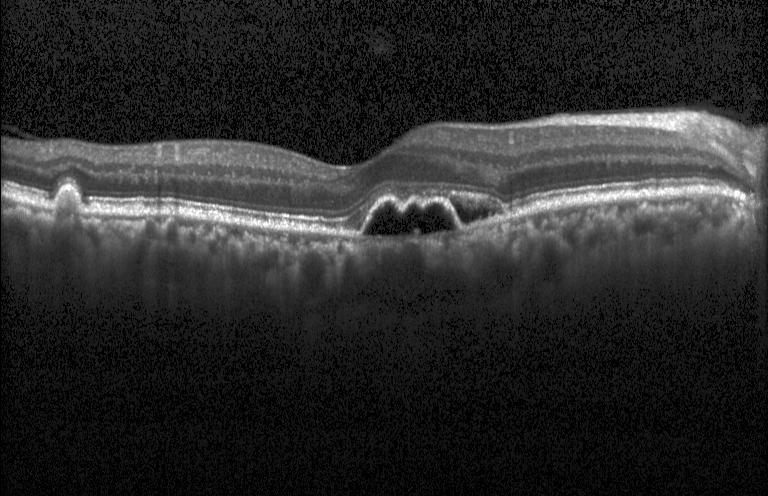

Macular scan; optical coherence tomography B-scan; instrument: Heidelberg Spectralis
Dx: a choroidal neovascular membrane.